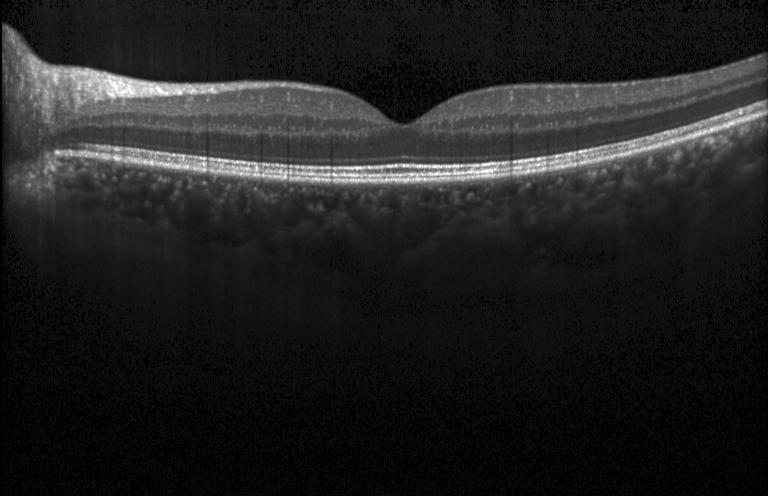

Instrument: Heidelberg Spectralis. Optical coherence tomography B-scan — This B-scan demonstrates no CNV, no DME, and no drusen.